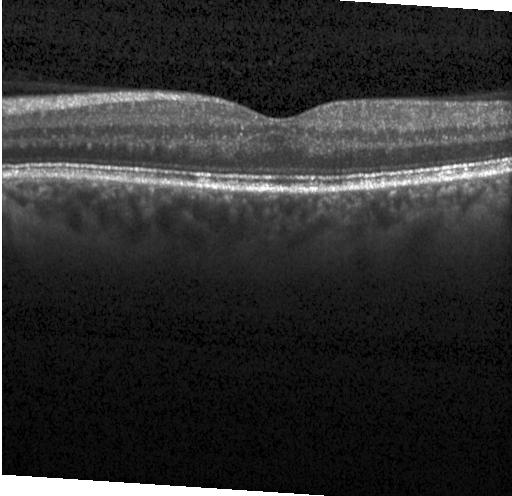 OCT B-scan — Finding: no CNV, no DME, and no drusen.